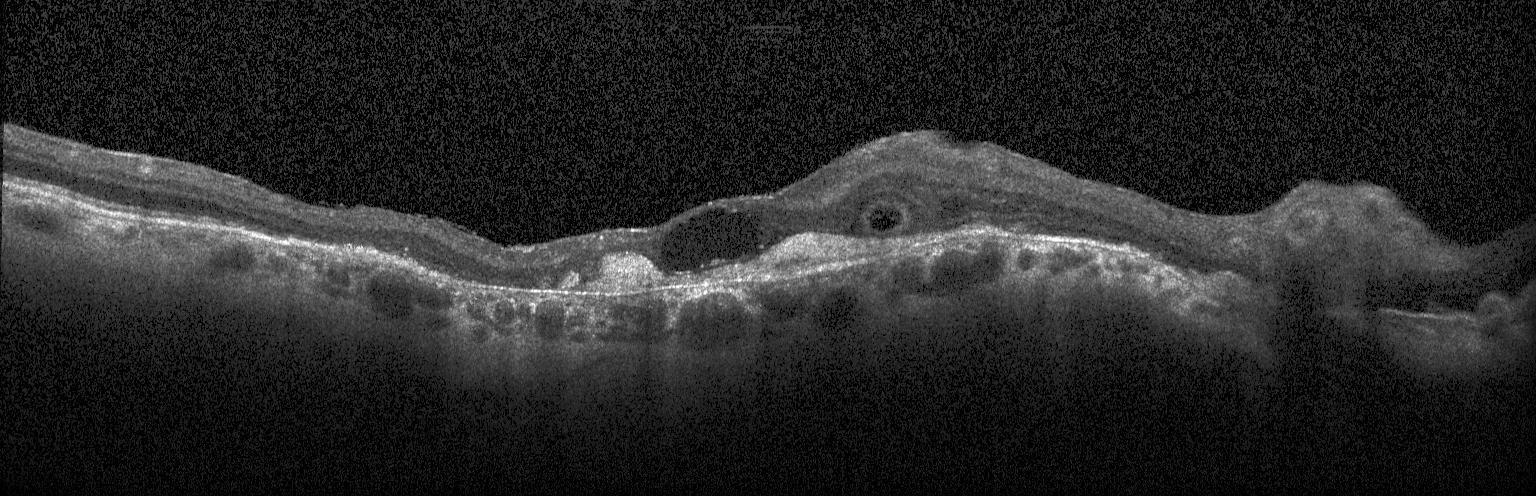
Finding: a choroidal neovascular membrane.